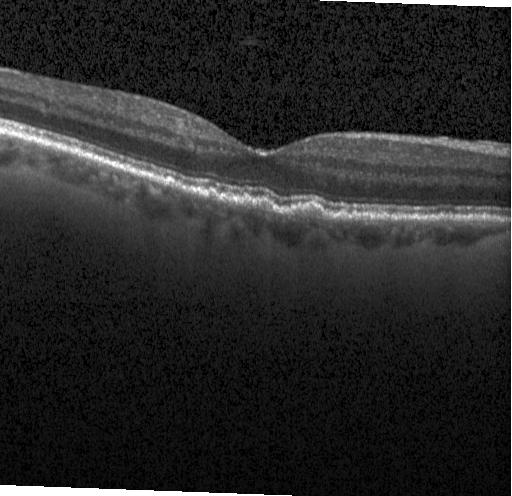 Spectral-domain OCT, through the macula, instrument: Heidelberg Spectralis, OCT B-scan.
The scan shows sub-RPE drusenoid deposits.